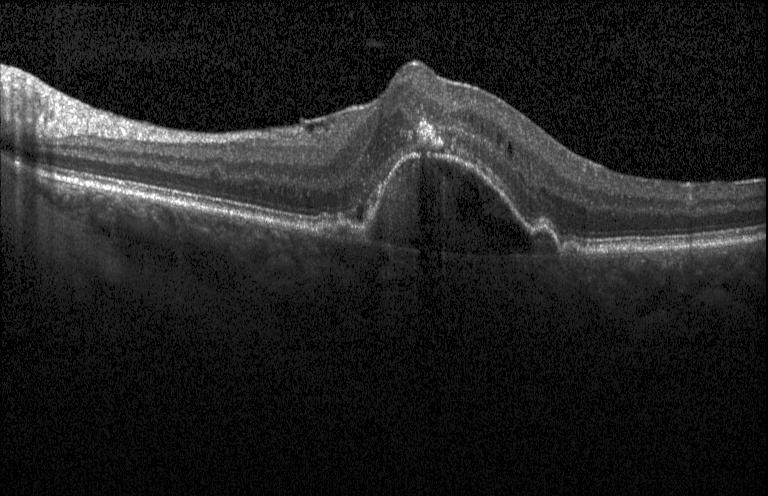 OCT line scan
Finding: CNV.